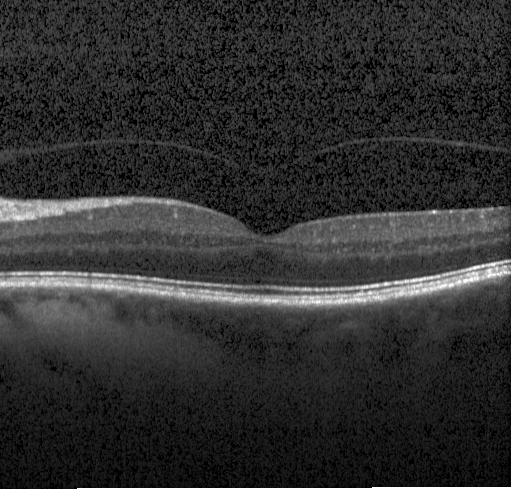

Macular scan, acquired on a Heidelberg Spectralis, spectral-domain OCT, OCT line scan — Assessment: neither choroidal neovascularization, diabetic macular edema, nor drusen.